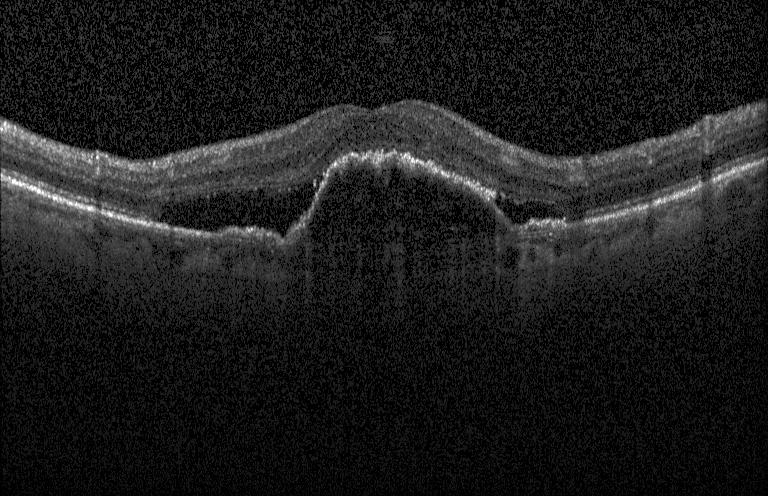 Dx: a choroidal neovascular membrane.